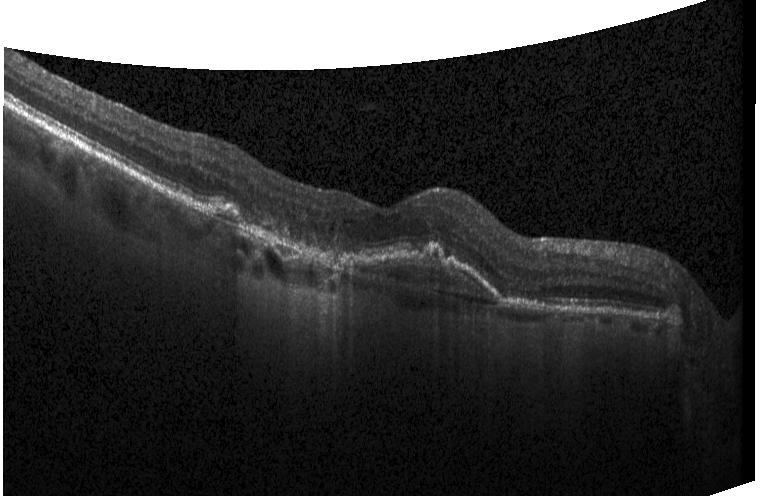
OCT B-scan.
Macular OCT: choroidal neovascularization.